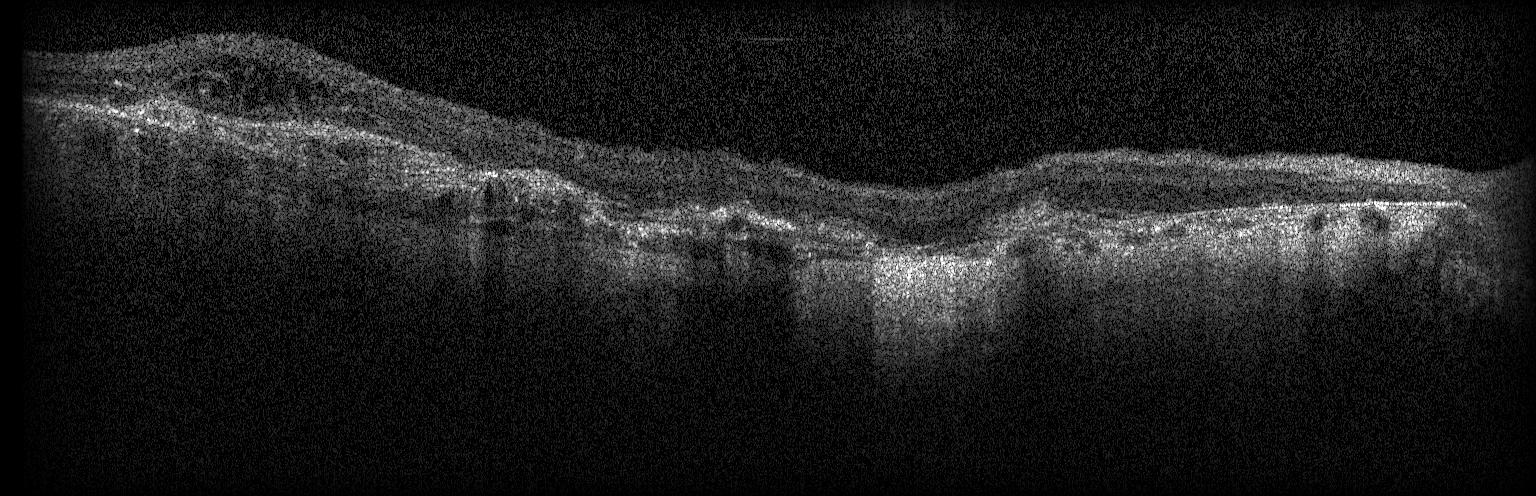
Retinal OCT B-scan · SD-OCT
Diagnosis: a choroidal neovascular membrane.